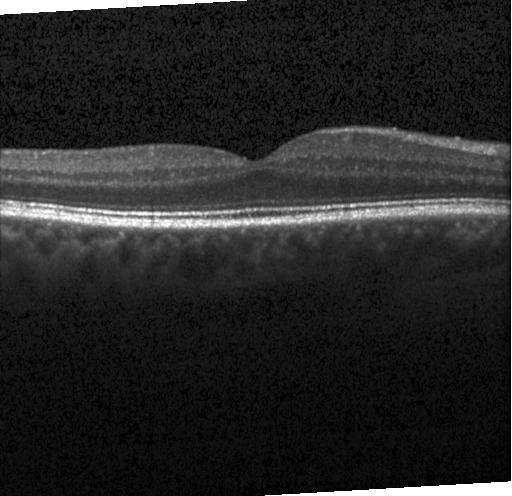

Optical coherence tomography scan
Dx: no choroidal neovascularization, diabetic macular edema, or drusen.